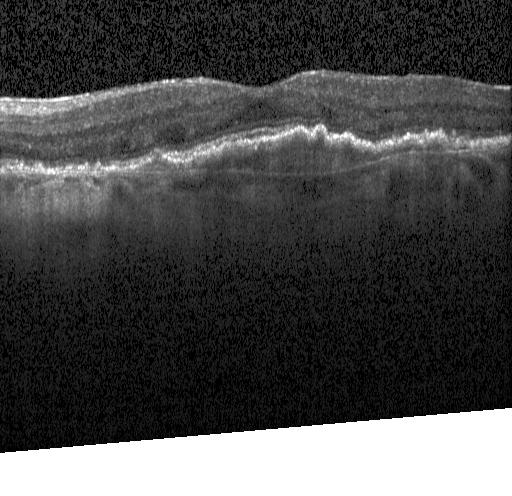 Finding: choroidal neovascularization.